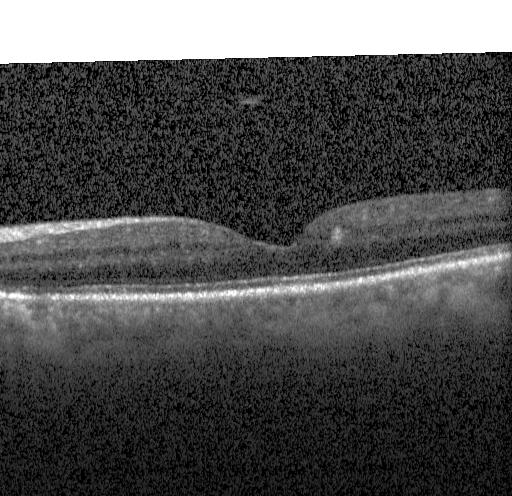

Retinal OCT B-scan, spectral-domain optical coherence tomography — Assessment: no choroidal neovascularization, diabetic macular edema, or drusen.